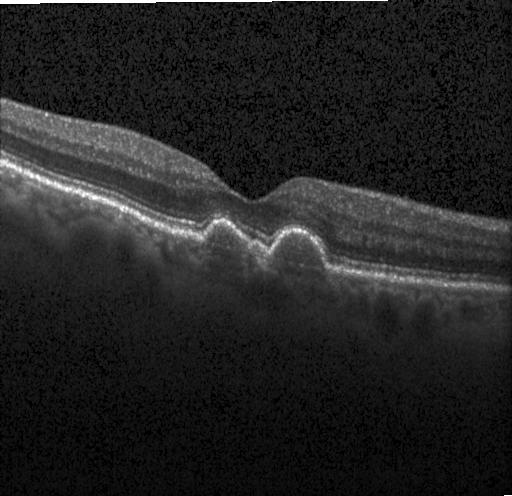

Spectral-domain OCT B-scan: drusen.